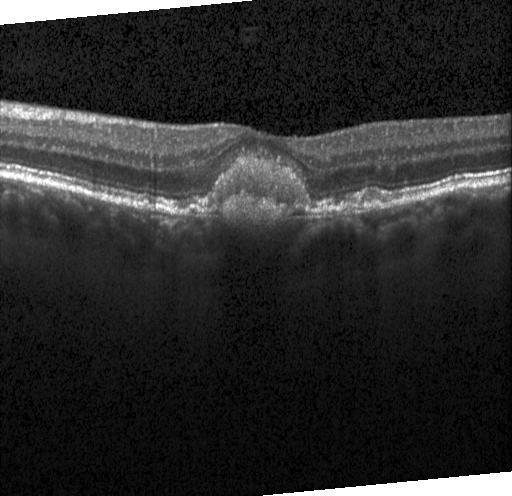 Optical coherence tomography scan — Impression: a choroidal neovascular membrane.